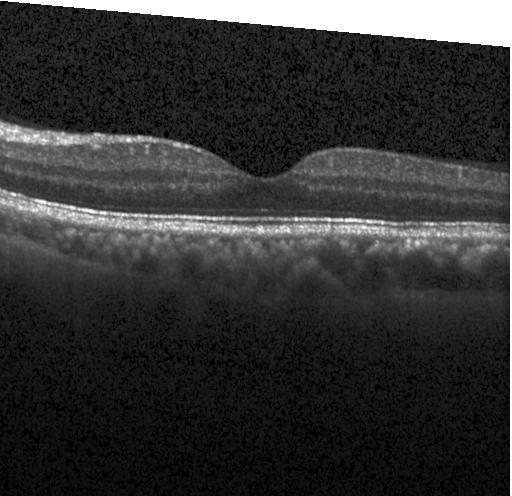

Finding: no CNV, no DME, and no drusen.